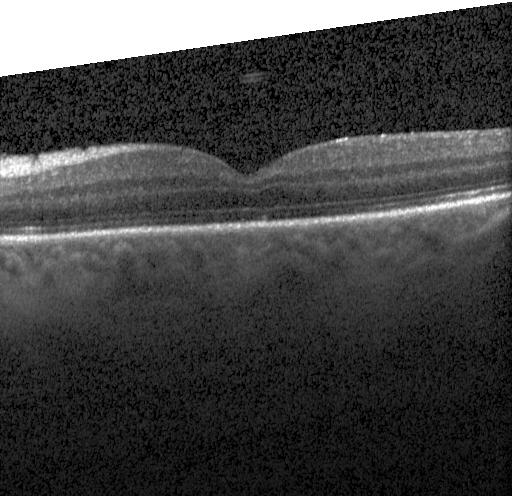 Diagnosis: no choroidal neovascularization, no diabetic macular edema, and no drusen.